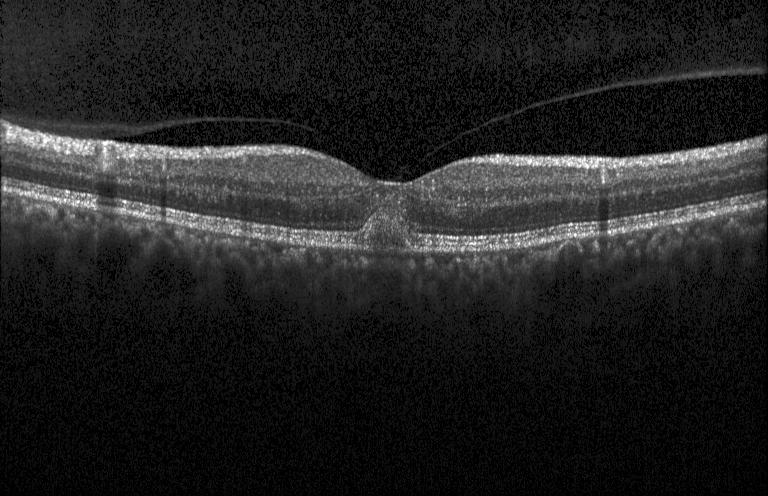
OCT finding: a choroidal neovascular membrane.